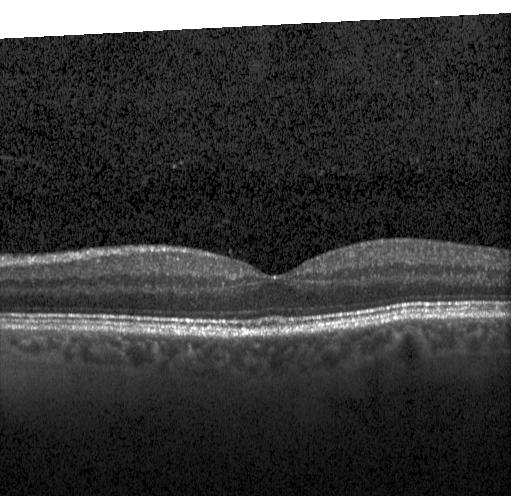
Finding: no CNV, no DME, and no drusen.